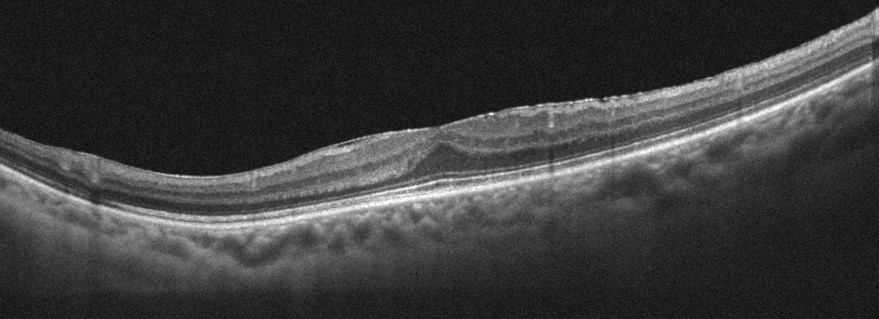 Retinal OCT cross-section — Dx: epiretinal membrane (ERM).